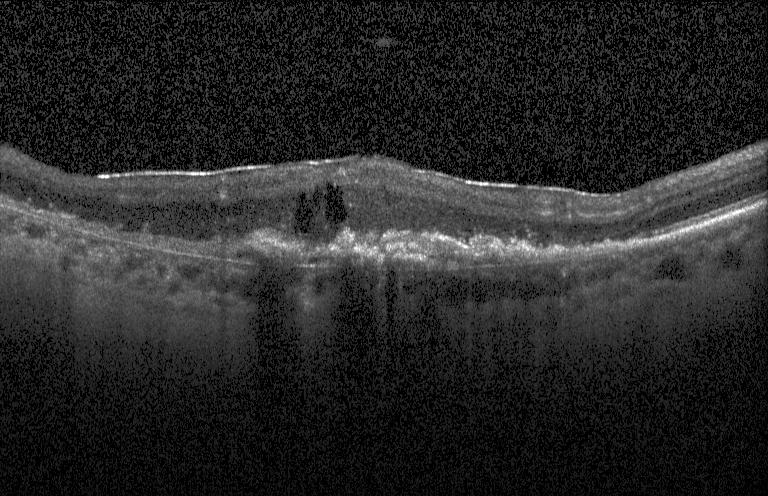 Optical coherence tomography scan, Heidelberg Spectralis
Choroidal neovascularization.